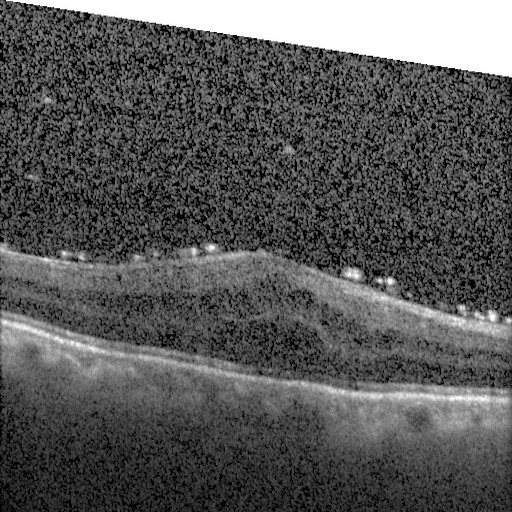

Acquired on a Heidelberg Spectralis · SD-OCT · OCT line scan. Impression: DME.